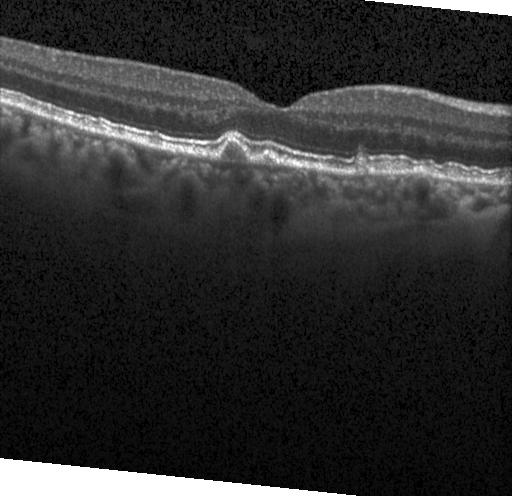
OCT line scan · Heidelberg Spectralis OCT system
Finding: sub-RPE drusenoid deposits.